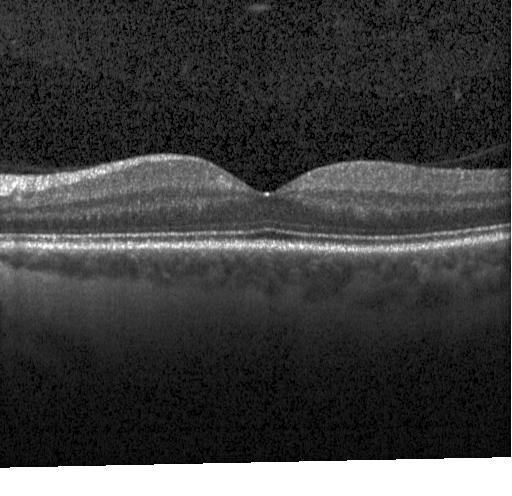
Impression: neither CNV, DME, nor drusen.